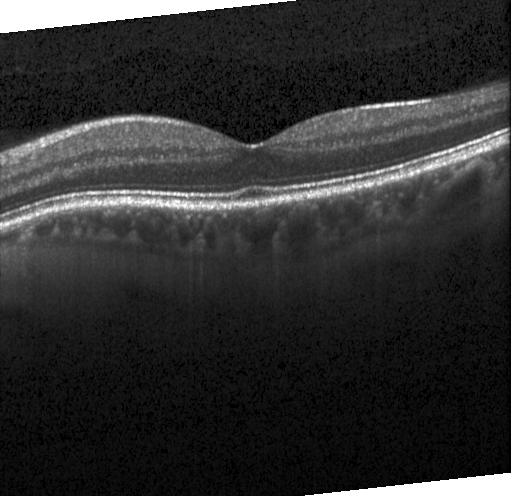
Finding: no choroidal neovascularization, diabetic macular edema, or drusen.